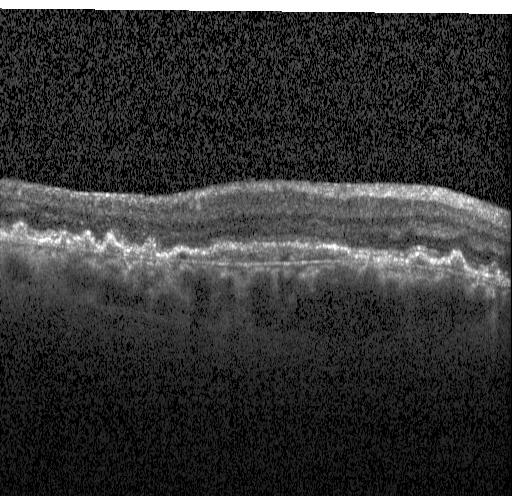 The scan shows a choroidal neovascular membrane.